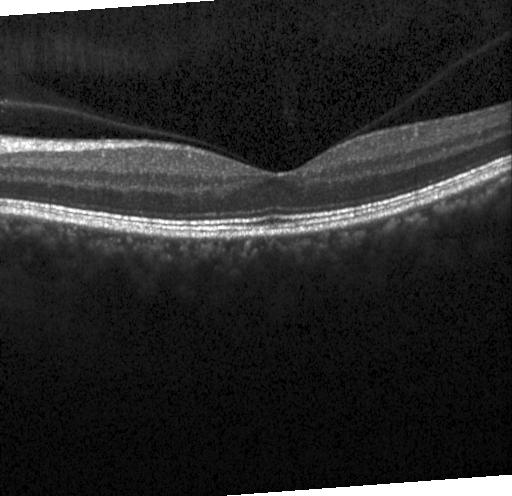 Optical coherence tomography B-scan, Heidelberg Spectralis OCT system, spectral-domain OCT, through the macula
Finding: no choroidal neovascularization, no diabetic macular edema, and no drusen.